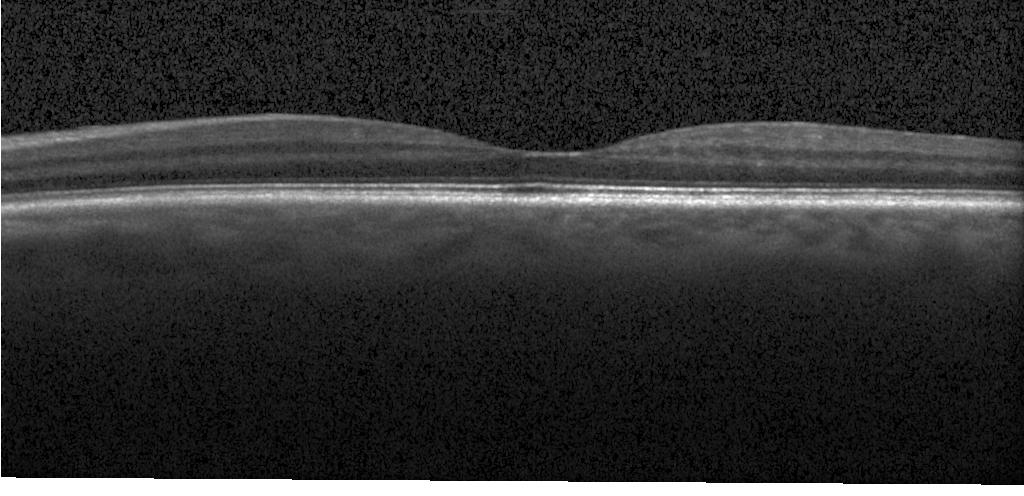

Instrument: Heidelberg Spectralis; spectral-domain OCT; horizontal scan through the fovea; optical coherence tomography scan — Macular OCT: neither CNV, DME, nor drusen.